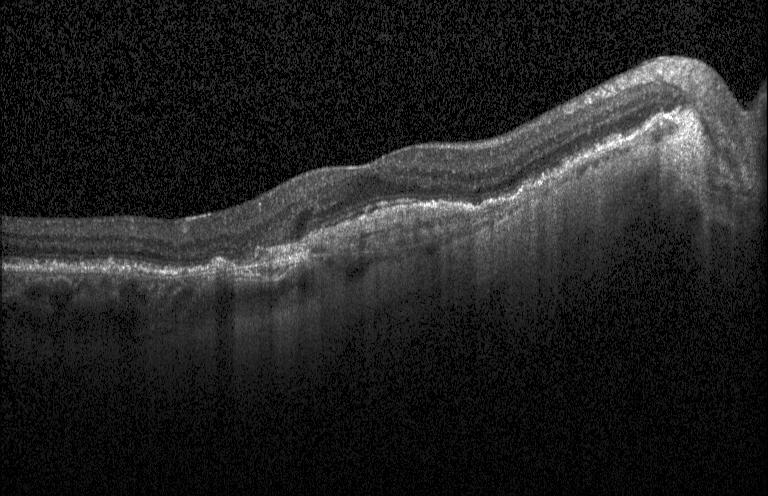 Horizontal scan through the fovea, instrument: Heidelberg Spectralis, retinal OCT cross-section.
Macular OCT: a choroidal neovascular membrane.